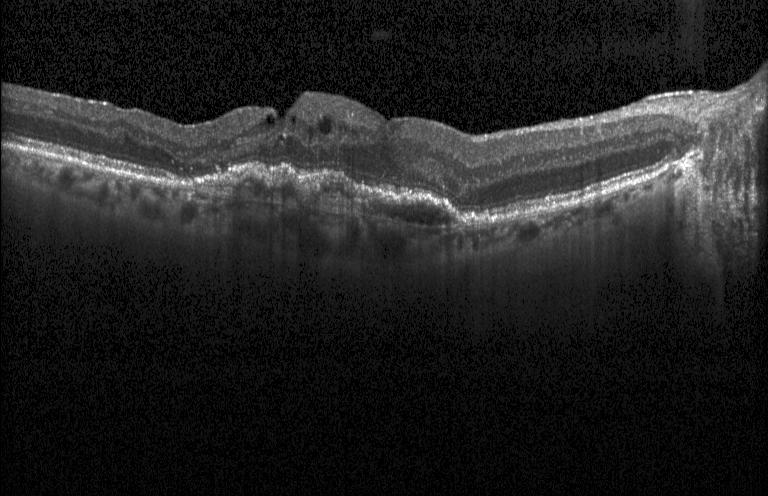

Finding: a choroidal neovascular membrane.